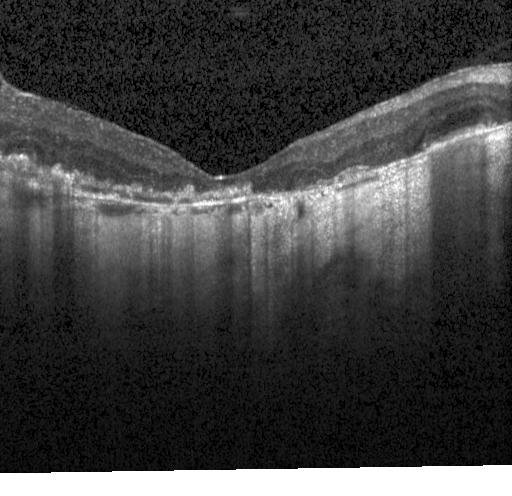
OCT scan showing a choroidal neovascular membrane.